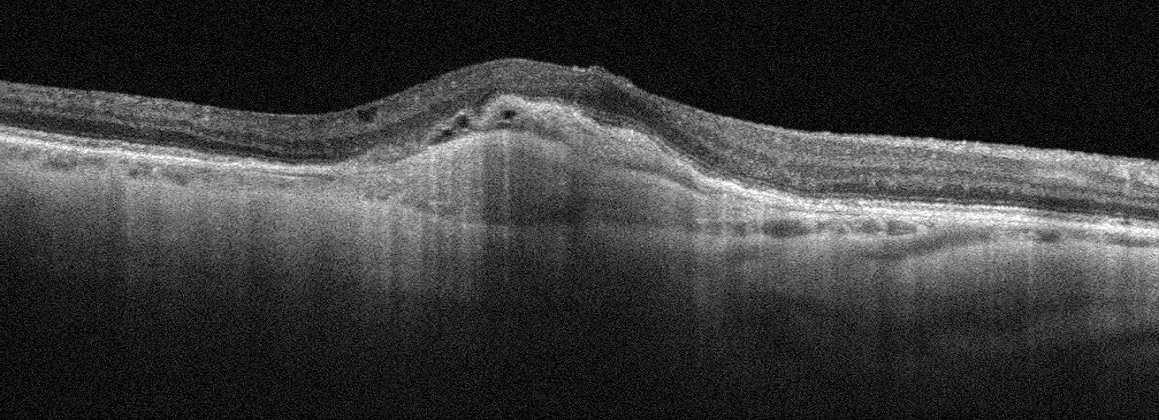 Optical coherence tomography scan · fovea-centered · instrument: Optovue Avanti RTVue XR · OS — Age-related macular degeneration.